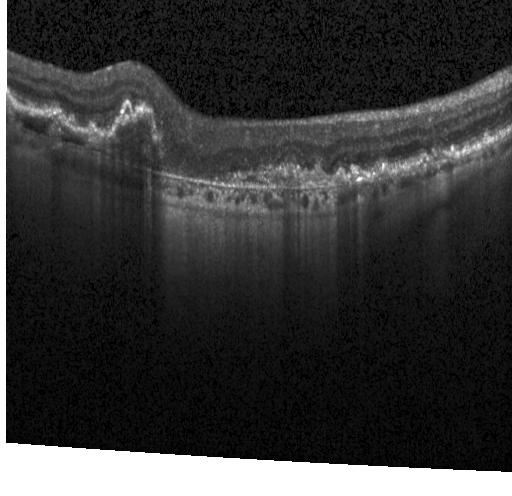

Retinal OCT cross-section
This B-scan demonstrates a choroidal neovascular membrane.